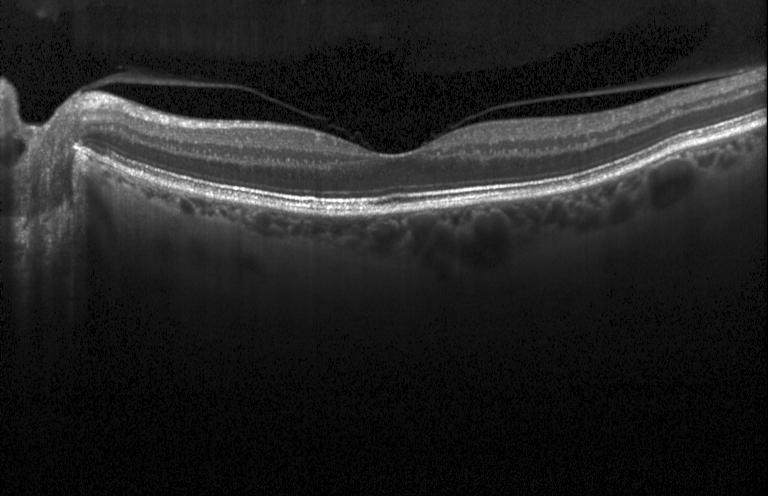
Acquired on a Heidelberg Spectralis. OCT B-scan. Impression: no choroidal neovascularization, diabetic macular edema, or drusen.